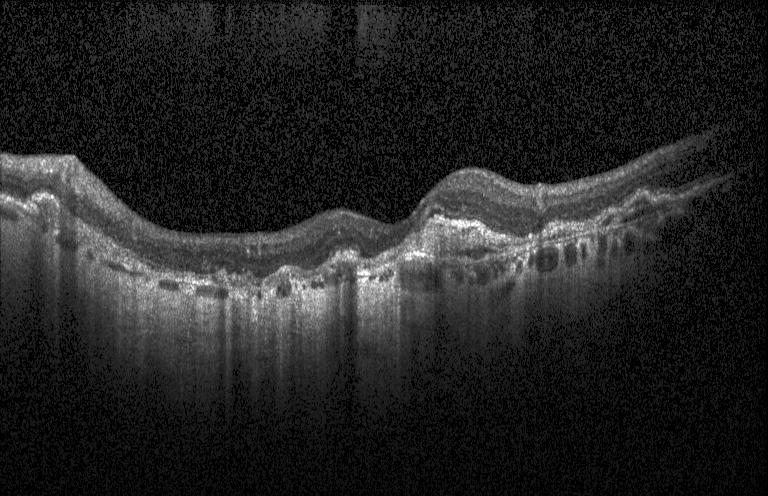

OCT B-scan showing choroidal neovascularization.